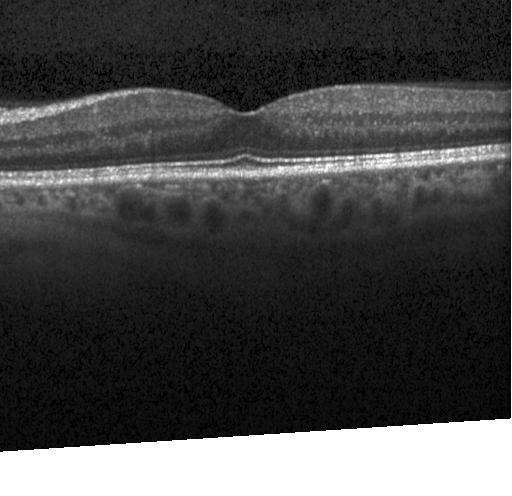 OCT B-scan, horizontal scan through the fovea, spectral-domain optical coherence tomography. OCT finding: neither CNV, DME, nor drusen.